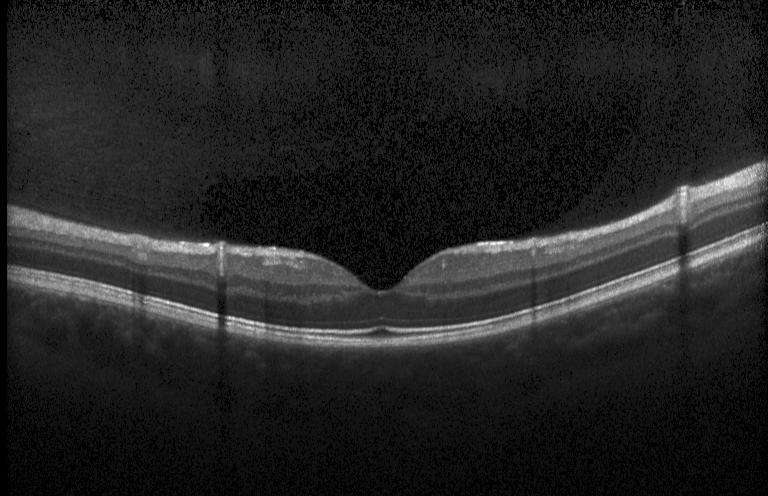 Acquired on a Heidelberg Spectralis. SD-OCT. Optical coherence tomography B-scan. Centered on the fovea — This B-scan demonstrates no CNV, DME, or drusen.